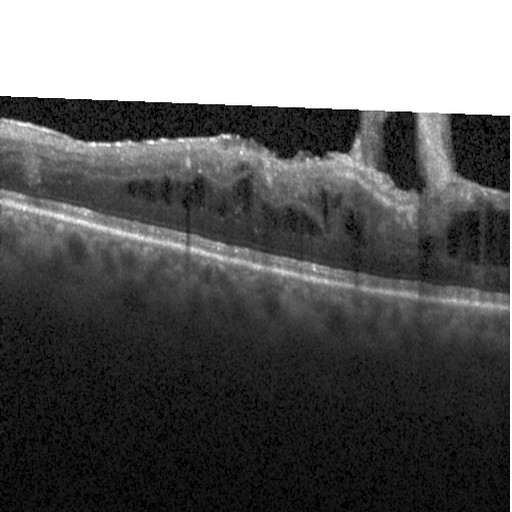

Finding: DME.